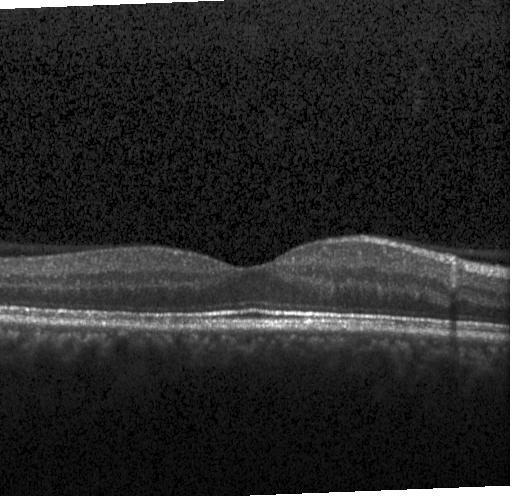
Retinal OCT B-scan, Heidelberg Spectralis OCT system. No choroidal neovascularization, no diabetic macular edema, and no drusen.